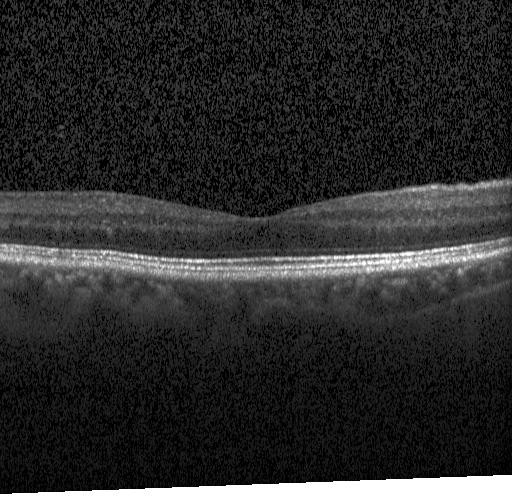

Finding: no choroidal neovascularization, no diabetic macular edema, and no drusen.